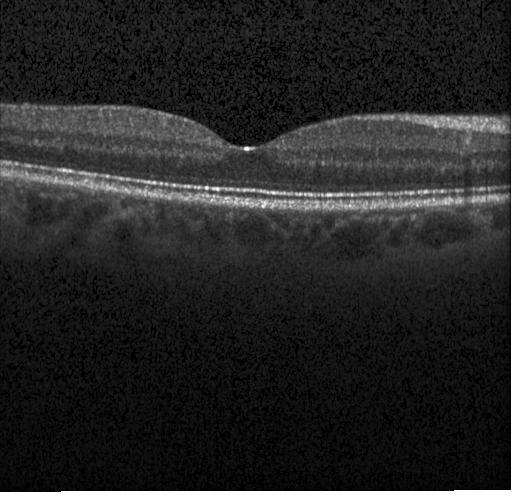
Optical coherence tomography B-scan. Centered on the fovea
Dx: no choroidal neovascularization, diabetic macular edema, or drusen.